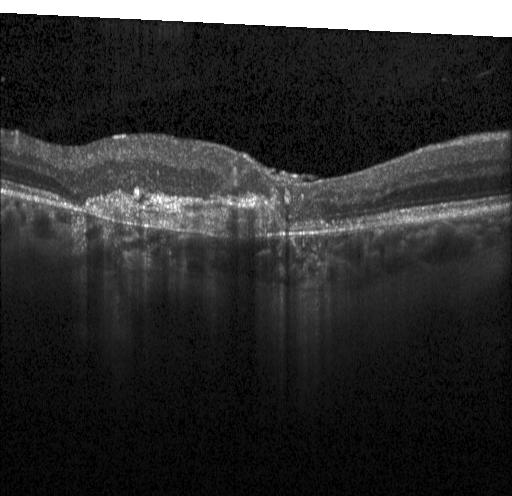 Heidelberg Spectralis OCT system, OCT line scan — Macular OCT: a choroidal neovascular membrane.